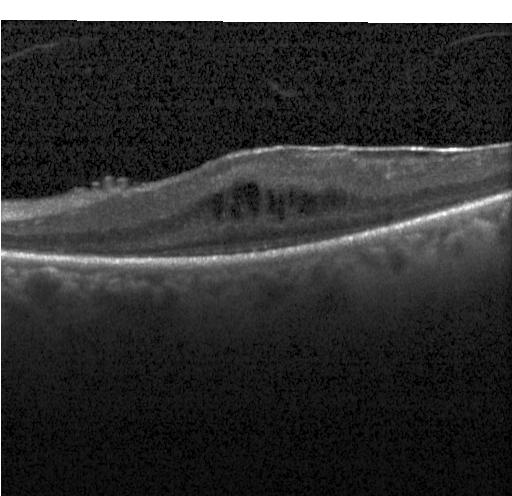 OCT line scan
Macular OCT: diabetic macular edema.